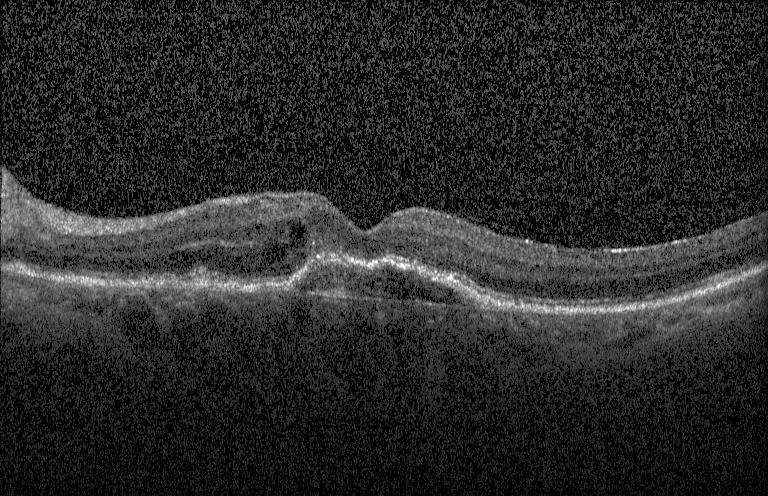 Instrument: Heidelberg Spectralis, spectral-domain optical coherence tomography, retinal OCT cross-section, fovea-centered.
Assessment: CNV.